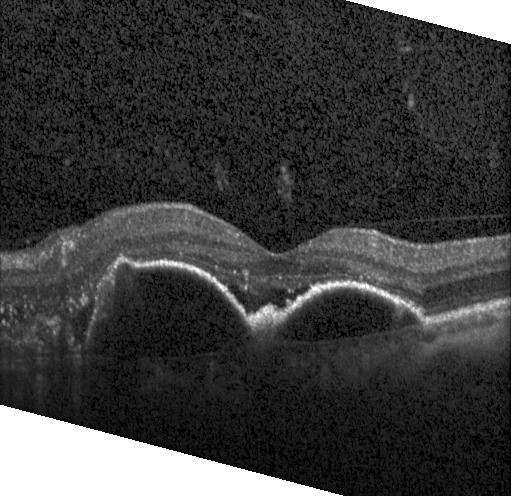
OCT B-scan. Spectral-domain optical coherence tomography.
Assessment: choroidal neovascularization.